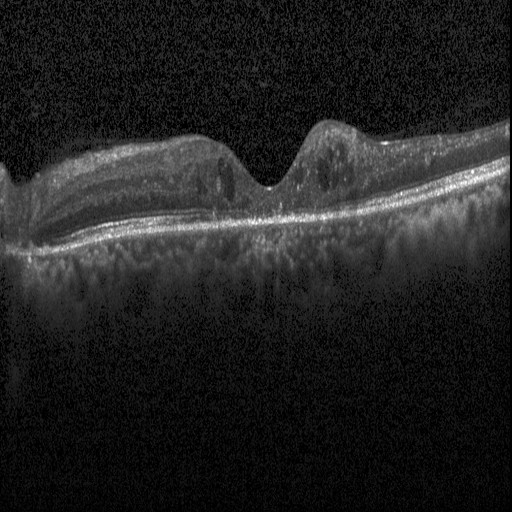

Macular OCT demonstrating diabetic macular edema (DME).